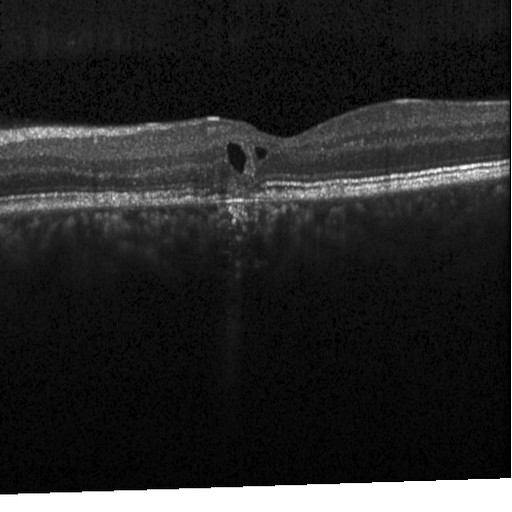
Retinal OCT cross-section — The scan shows diabetic macular edema.